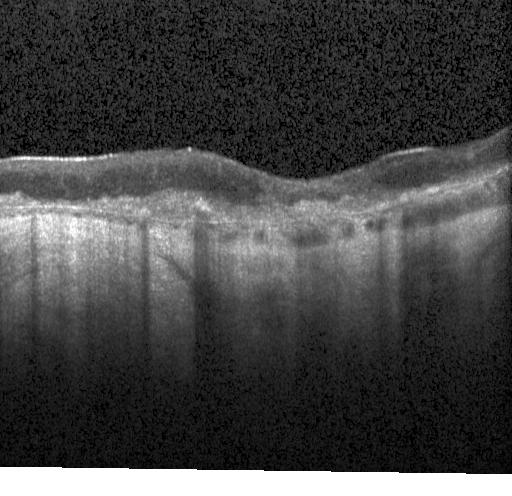 Impression: choroidal neovascularization (CNV).